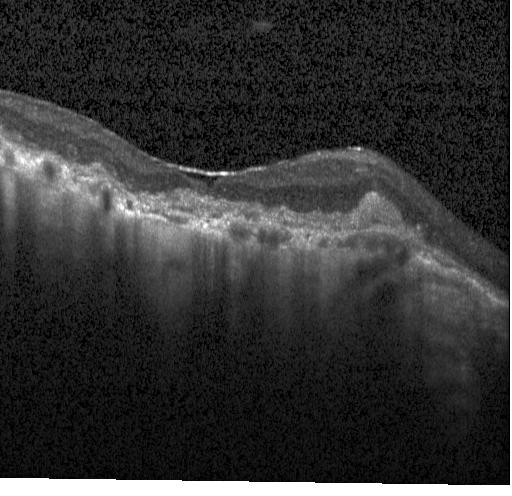

Impression: a choroidal neovascular membrane.